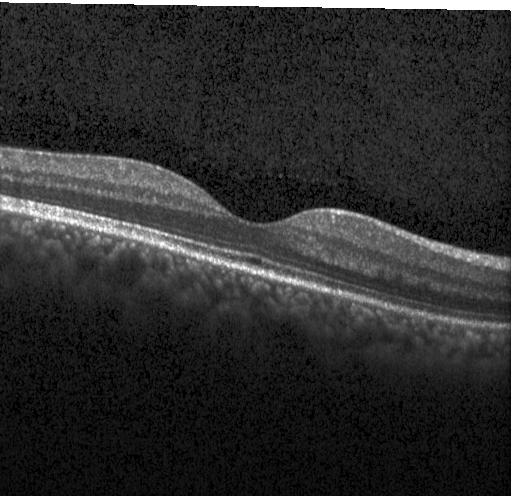 Optical coherence tomography scan.
This B-scan demonstrates no CNV, DME, or drusen.